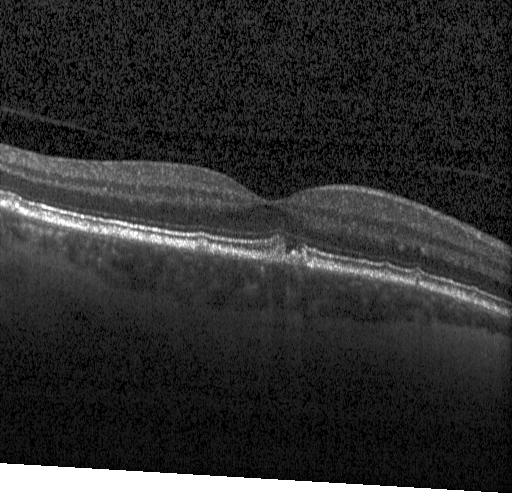

Optical coherence tomography scan · macular scan.
Assessment: sub-RPE drusenoid deposits.